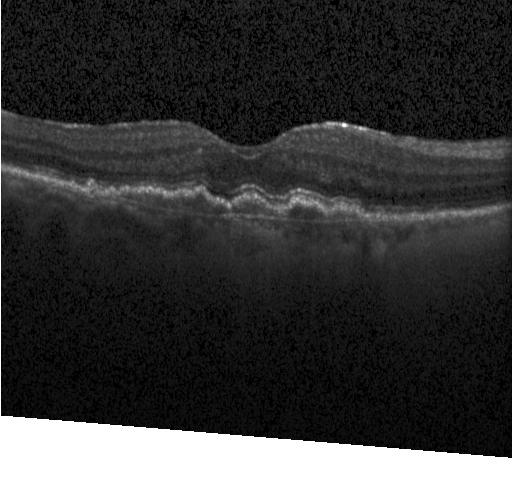

Optical coherence tomography B-scan. Instrument: Heidelberg Spectralis.
Diagnosis: a choroidal neovascular membrane.